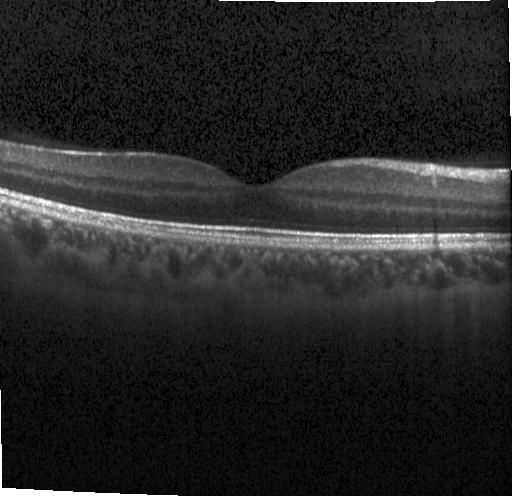
SD-OCT · acquired on a Heidelberg Spectralis · horizontal scan through the fovea · retinal OCT cross-section.
Macular OCT: neither choroidal neovascularization, diabetic macular edema, nor drusen.